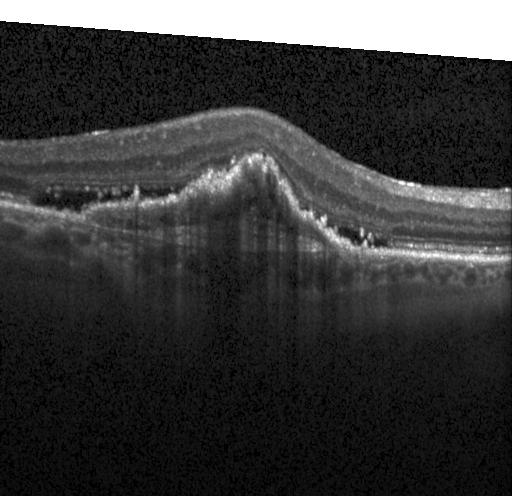

Impression: a choroidal neovascular membrane.